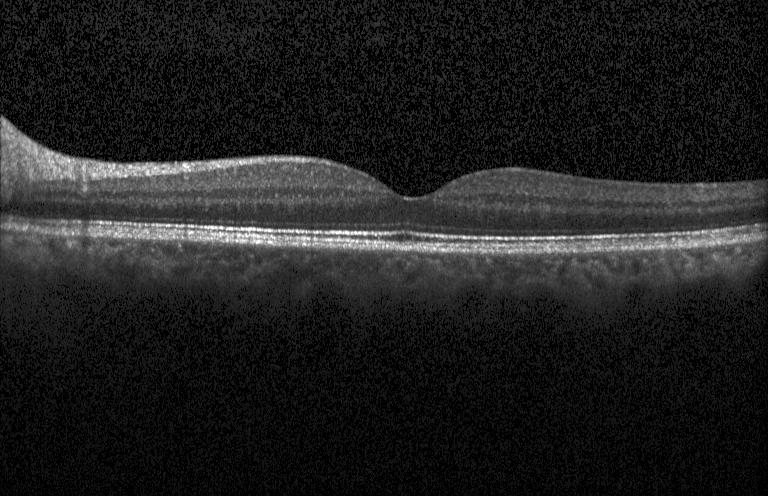
Fovea-centered; instrument: Heidelberg Spectralis; optical coherence tomography scan; spectral-domain optical coherence tomography — Diagnosis: neither choroidal neovascularization, diabetic macular edema, nor drusen.